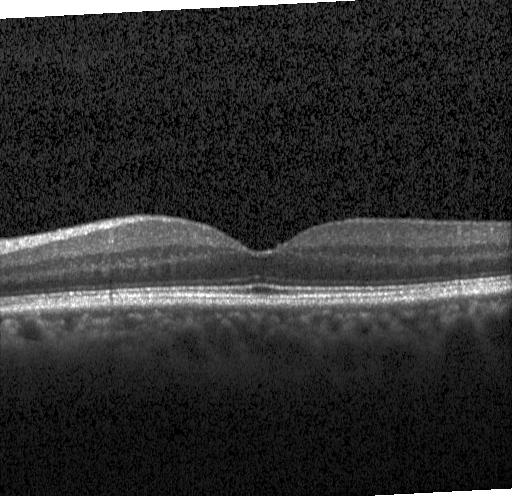
Retinal OCT cross-section.
The scan shows neither CNV, DME, nor drusen.